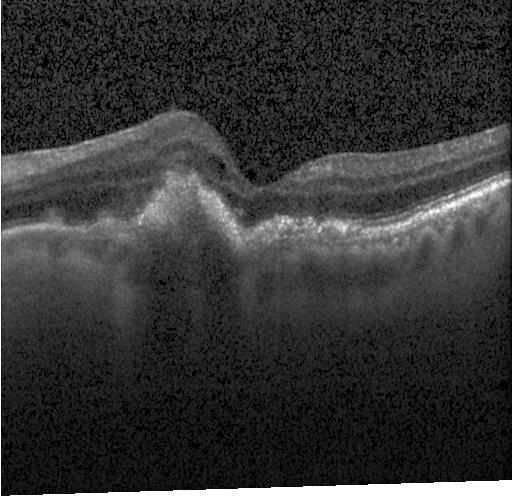
Spectral-domain OCT, instrument: Heidelberg Spectralis, OCT B-scan
This B-scan demonstrates a choroidal neovascular membrane.